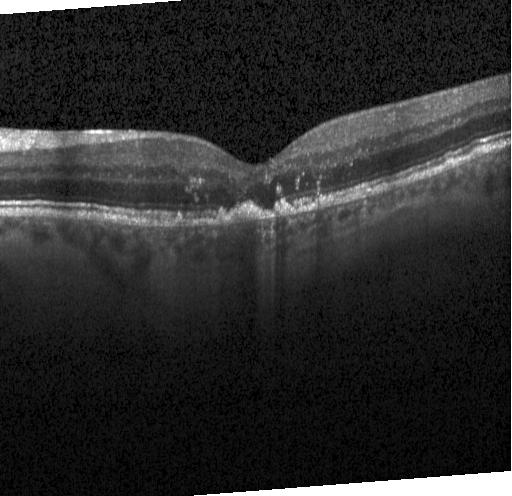

Diagnosis: a choroidal neovascular membrane.